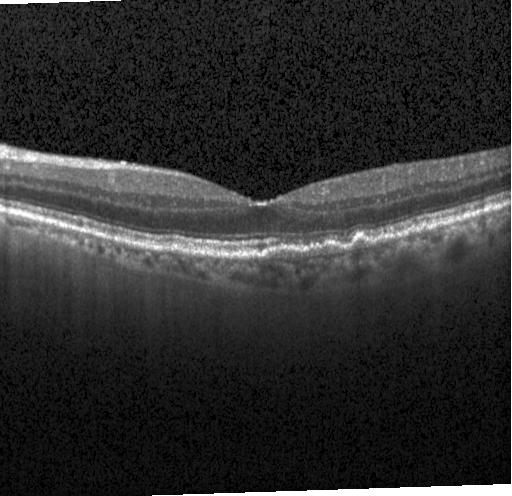
OCT B-scan.
Impression: multiple drusen.